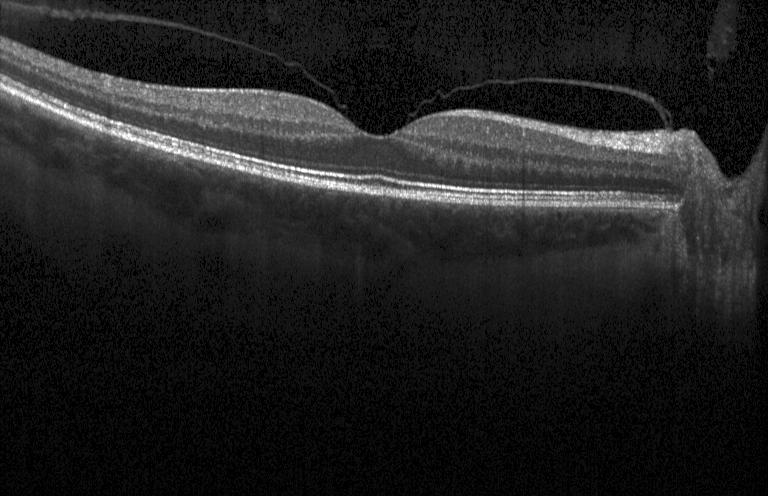
Through the macula, optical coherence tomography scan, spectral-domain OCT. Macular OCT: no choroidal neovascularization, diabetic macular edema, or drusen.